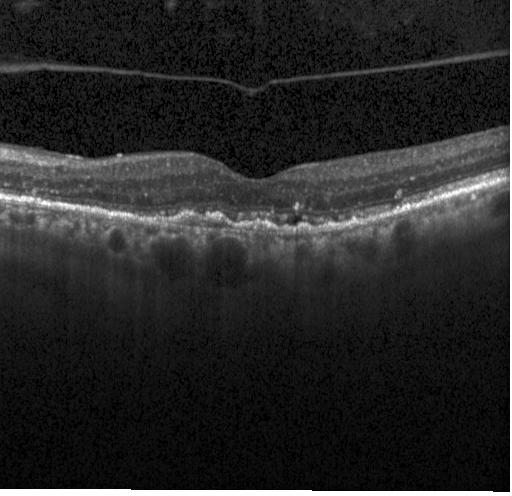

Dx: a choroidal neovascular membrane.